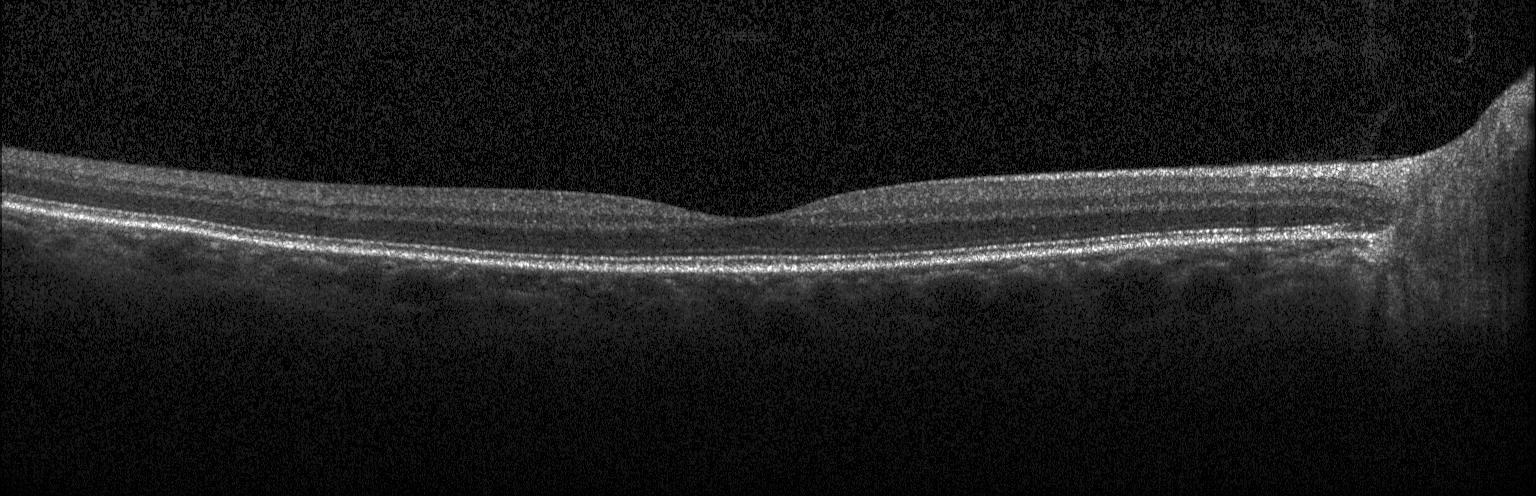

Assessment: no evidence of CNV, DME, or drusen.